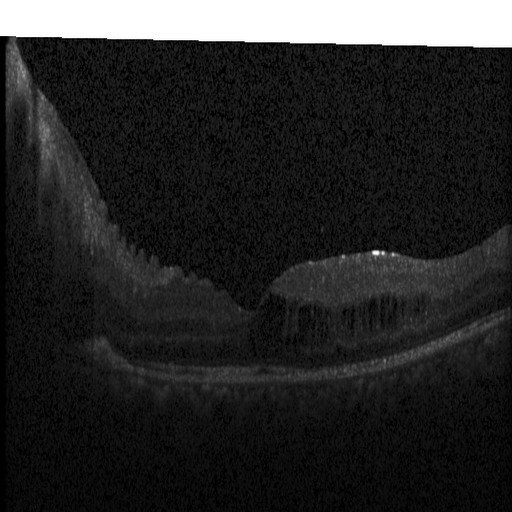
Retinal OCT B-scan — Impression: DME.